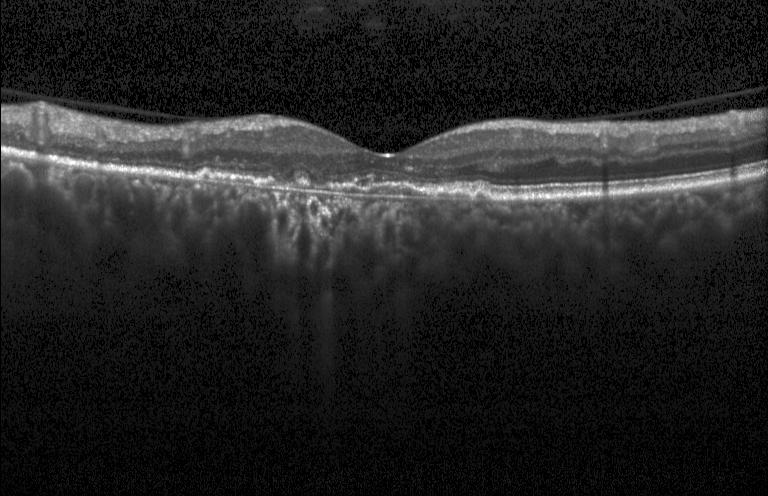 OCT line scan — This B-scan demonstrates a choroidal neovascular membrane.